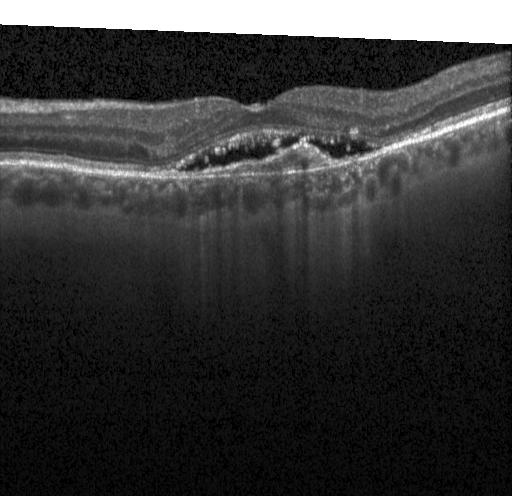

Impression: choroidal neovascularization.